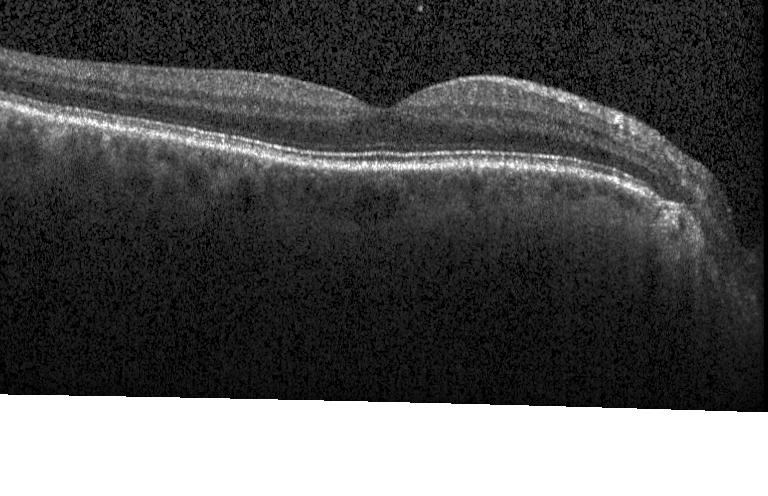

OCT line scan; fovea-centered. Finding: neither CNV, DME, nor drusen.